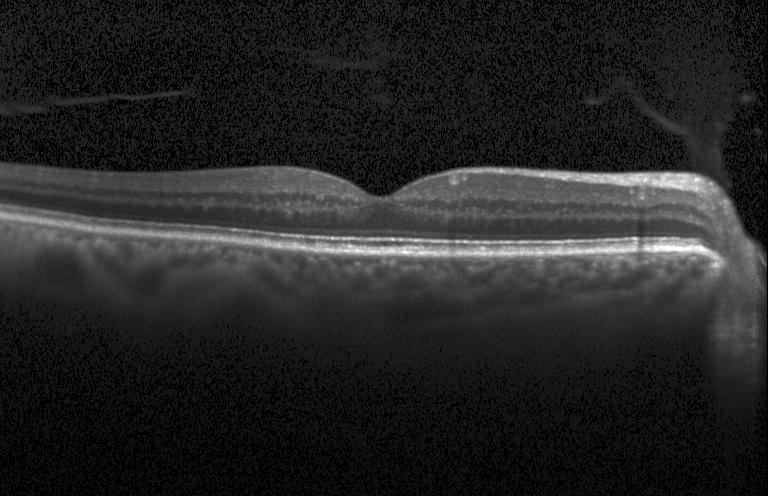

Instrument: Heidelberg Spectralis; optical coherence tomography B-scan; spectral-domain optical coherence tomography. Diagnosis: no evidence of choroidal neovascularization, diabetic macular edema, or drusen.